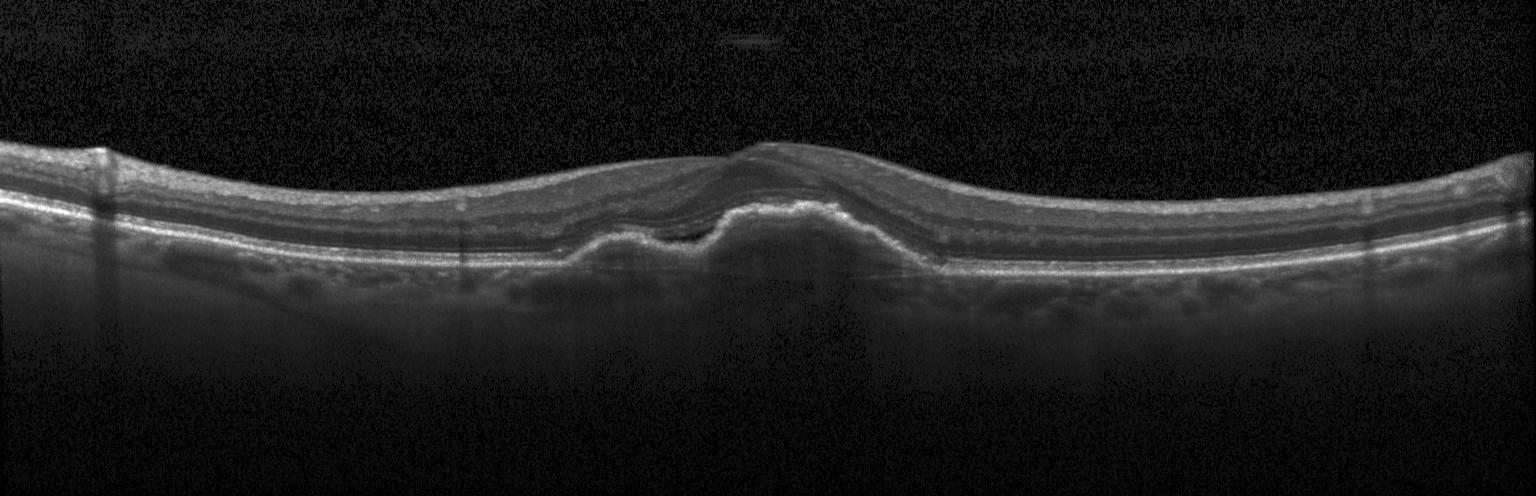 Finding: CNV.